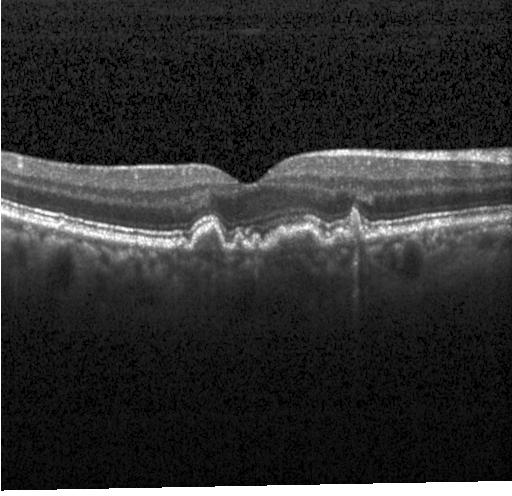 OCT line scan. Instrument: Heidelberg Spectralis. Horizontal scan through the fovea. Diagnosis: drusen.